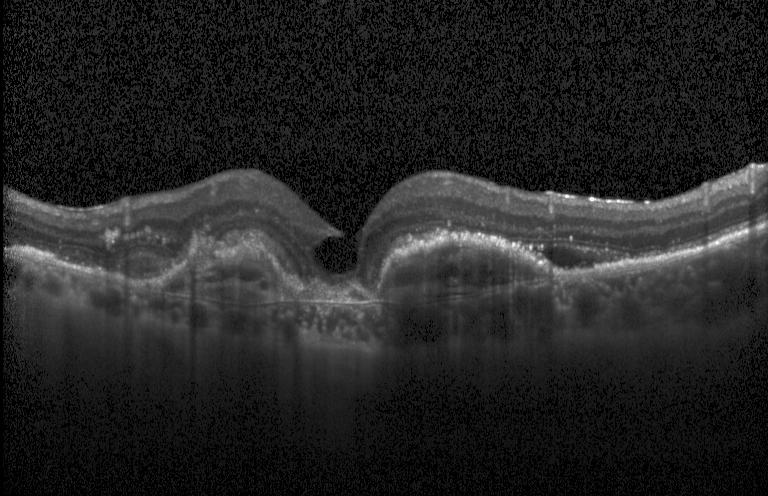 Optical coherence tomography B-scan
Diagnosis: choroidal neovascularization (CNV).